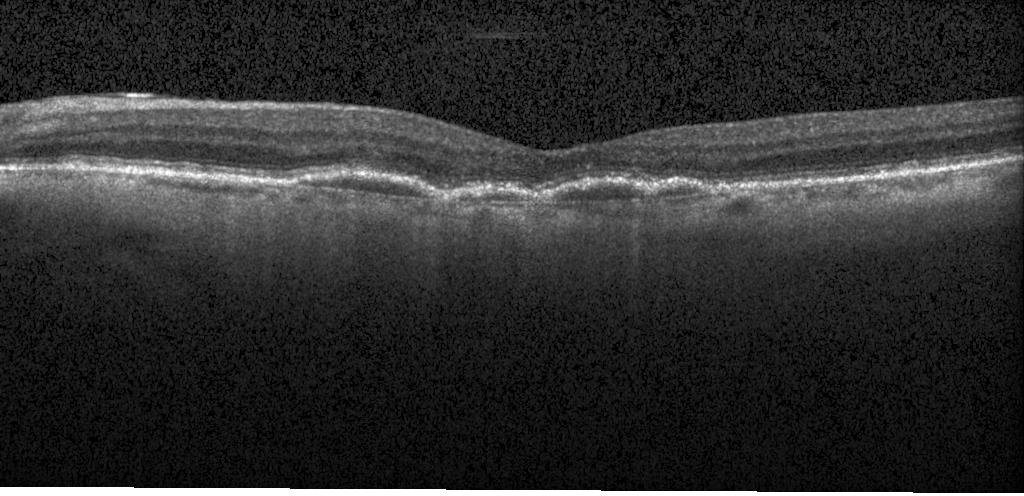

Retinal OCT cross-section showing a choroidal neovascular membrane.